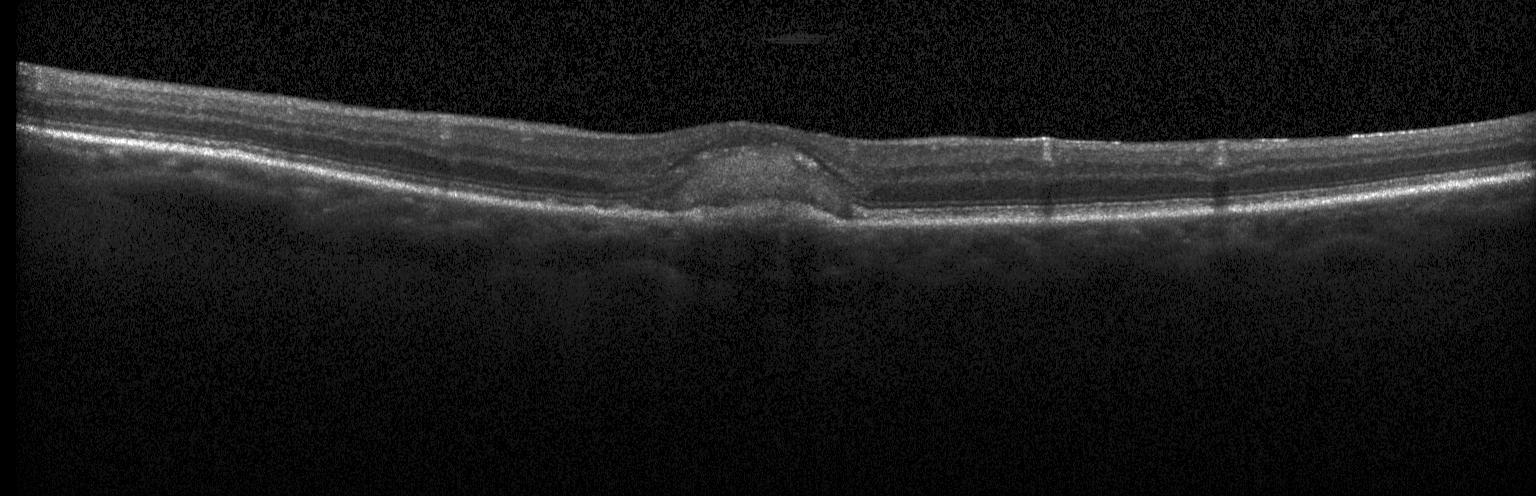

Diagnosis: CNV.